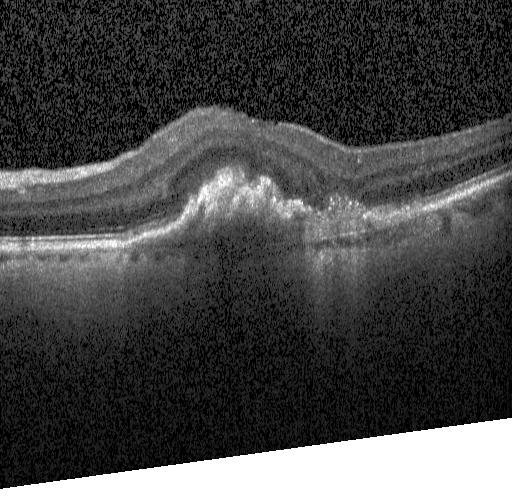 OCT B-scan · acquired on a Heidelberg Spectralis
OCT finding: choroidal neovascularization.